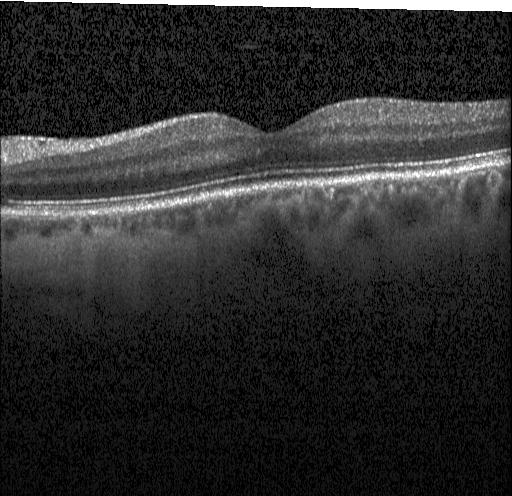 Through the macula; retinal OCT cross-section; spectral-domain optical coherence tomography; Heidelberg Spectralis OCT system — Impression: no evidence of choroidal neovascularization, diabetic macular edema, or drusen.